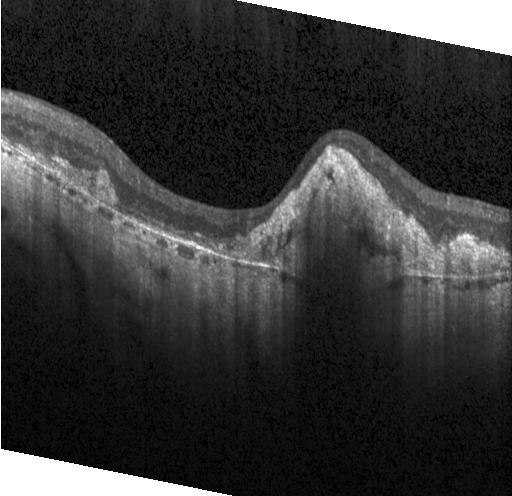
Heidelberg Spectralis, centered on the fovea, spectral-domain OCT, optical coherence tomography B-scan — Diagnosis: choroidal neovascularization.